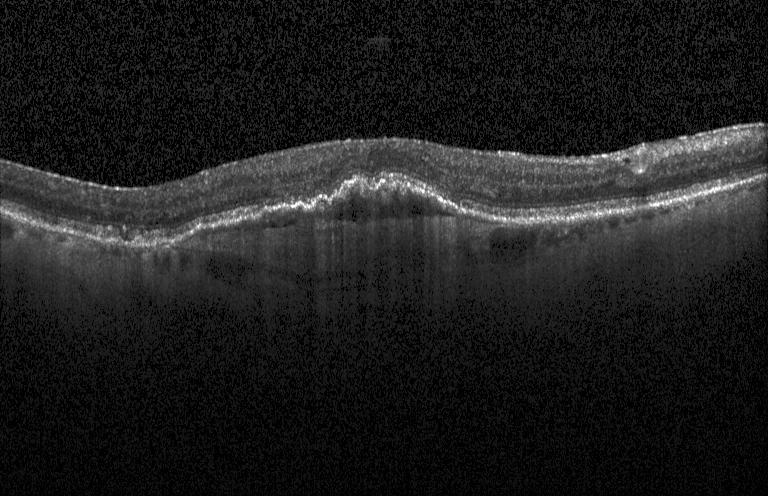

OCT B-scan · Heidelberg Spectralis OCT system.
Impression: a choroidal neovascular membrane.